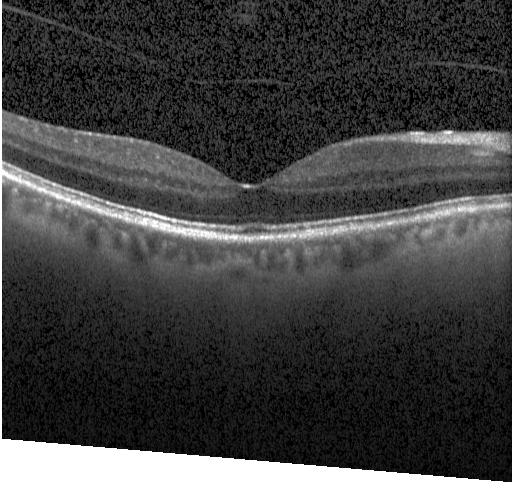

Retinal OCT B-scan. SD-OCT. This B-scan demonstrates no evidence of CNV, DME, or drusen.